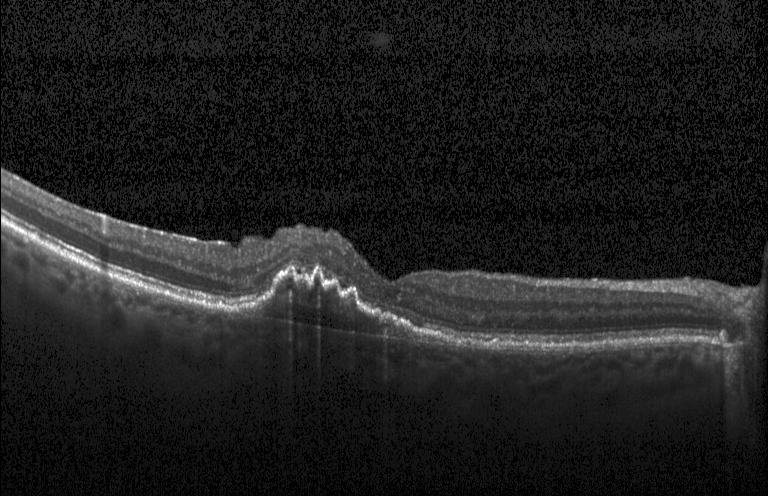
Finding: choroidal neovascularization (CNV).